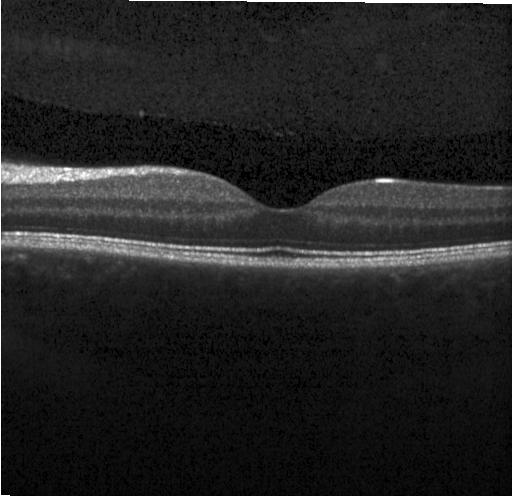

Impression: neither choroidal neovascularization, diabetic macular edema, nor drusen.